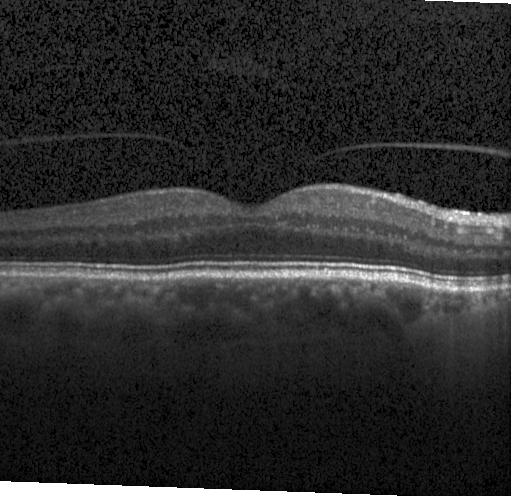 Optical coherence tomography B-scan. OCT finding: no choroidal neovascularization, no diabetic macular edema, and no drusen.